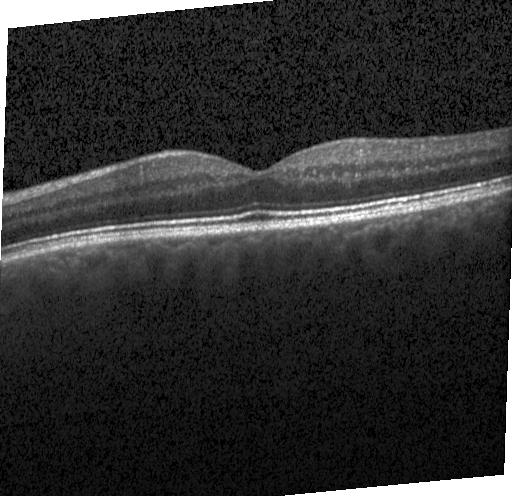
Macular OCT: no choroidal neovascularization, no diabetic macular edema, and no drusen.